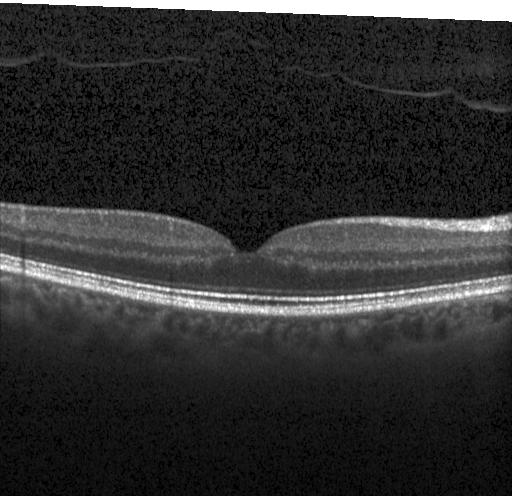 Horizontal scan through the fovea. Spectral-domain optical coherence tomography. Optical coherence tomography B-scan. Heidelberg Spectralis OCT system — Macular OCT: no choroidal neovascularization, diabetic macular edema, or drusen.